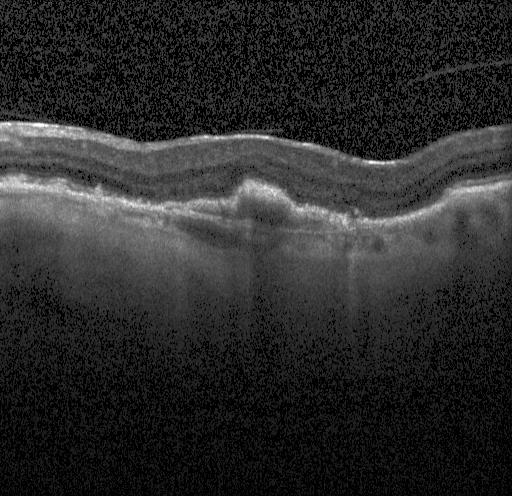 Instrument: Heidelberg Spectralis · retinal OCT B-scan
Diagnosis: choroidal neovascularization.